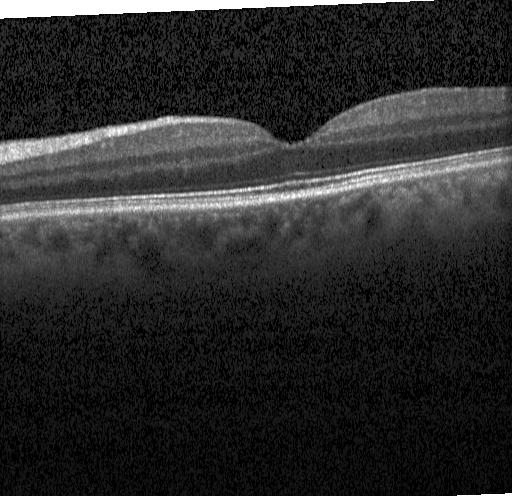
Spectral-domain OCT. OCT B-scan. Heidelberg Spectralis
Diagnosis: neither choroidal neovascularization, diabetic macular edema, nor drusen.